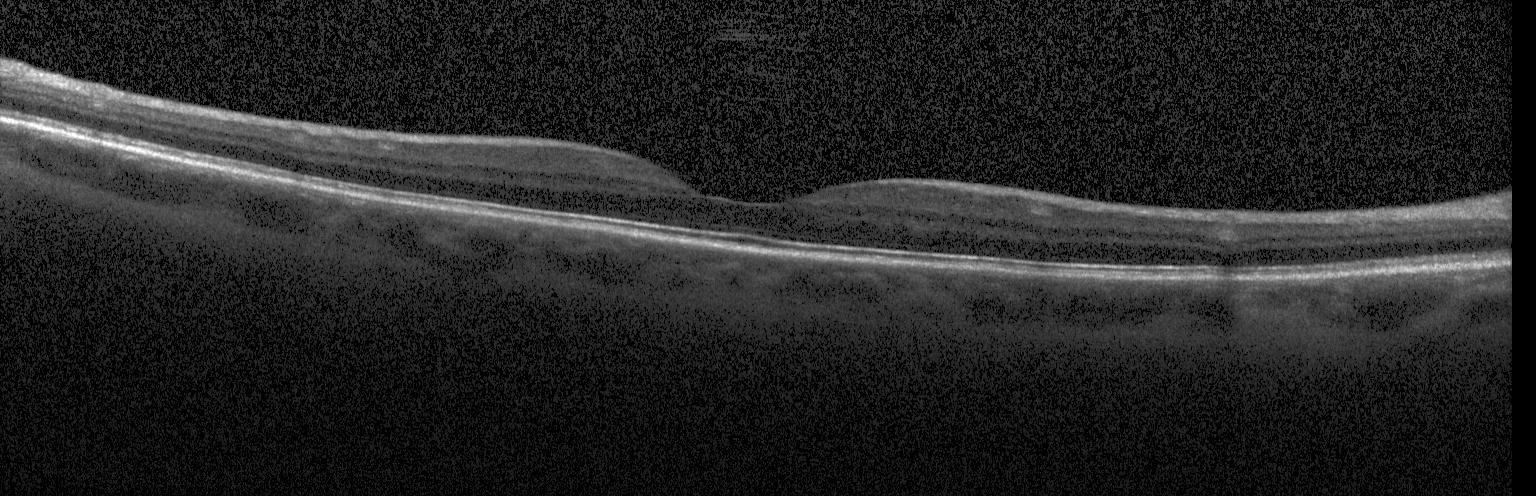
Optical coherence tomography B-scan — OCT finding: no evidence of choroidal neovascularization, diabetic macular edema, or drusen.